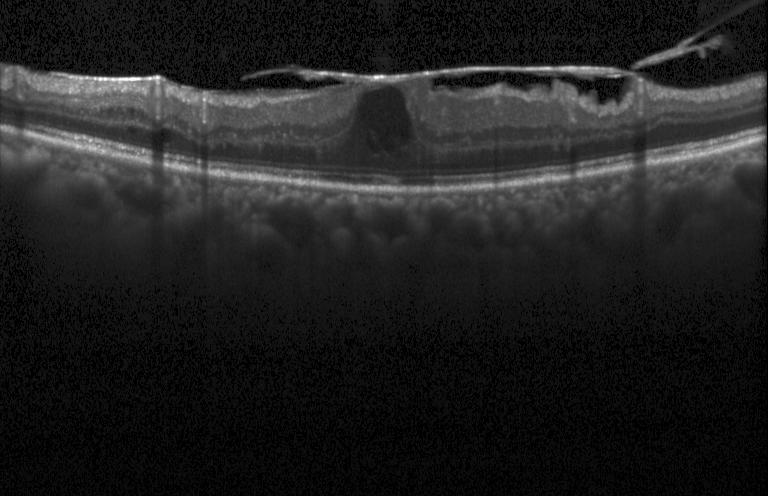 Through the macula; SD-OCT; retinal OCT B-scan.
DME.